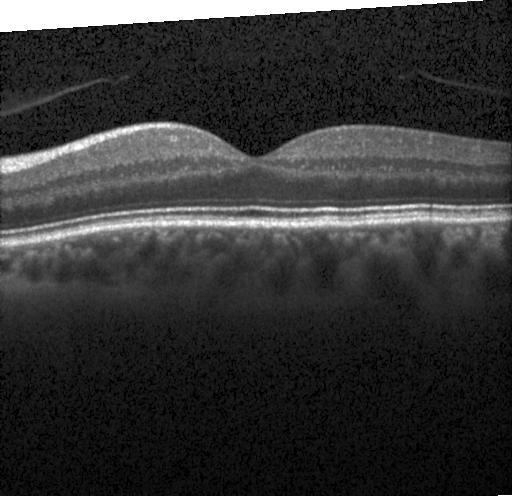

Impression: neither choroidal neovascularization, diabetic macular edema, nor drusen.